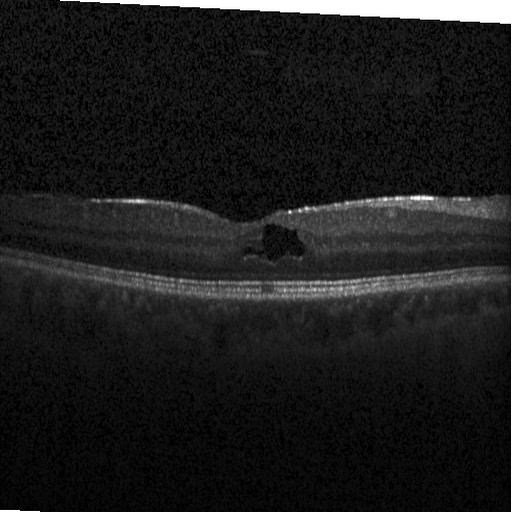

Heidelberg Spectralis OCT system. OCT B-scan. Macular scan
The scan shows diabetic macular edema.